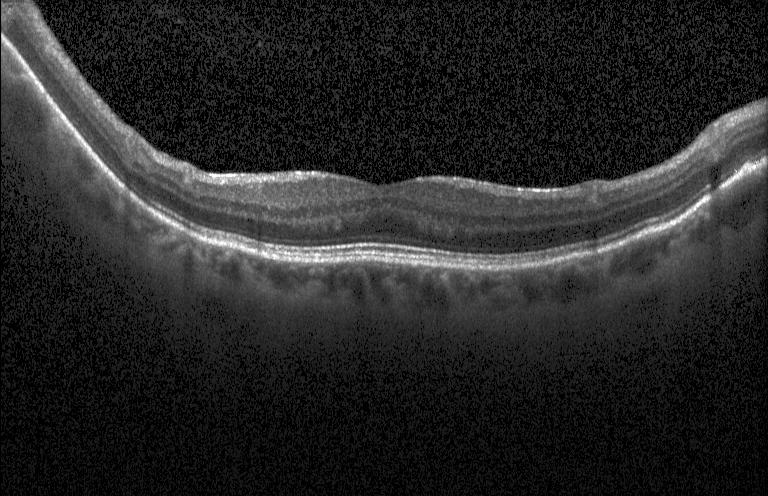
Retinal OCT B-scan · SD-OCT · Heidelberg Spectralis · fovea-centered. Neither CNV, DME, nor drusen.